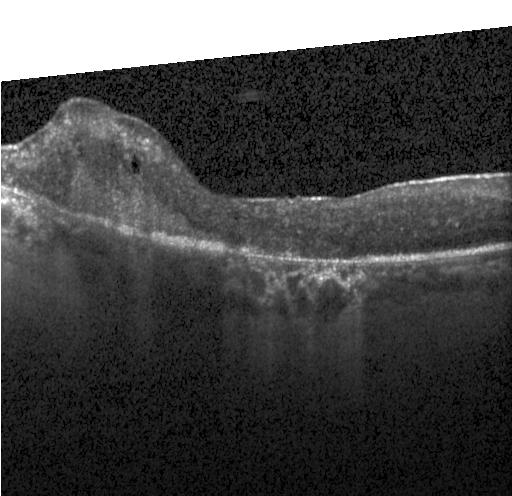

Acquired on a Heidelberg Spectralis, SD-OCT, optical coherence tomography B-scan. Finding: choroidal neovascularization.